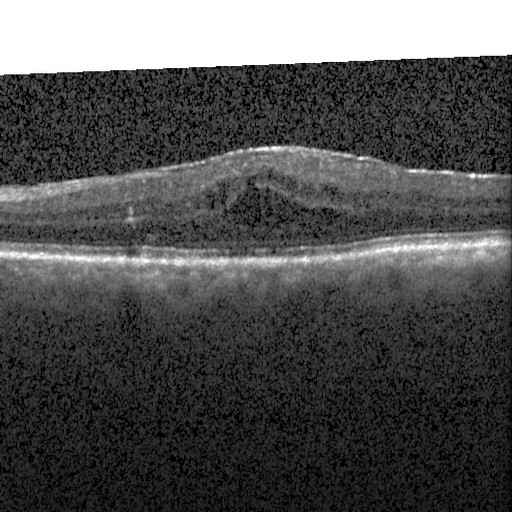 Retinal OCT cross-section. Assessment: diabetic macular edema.